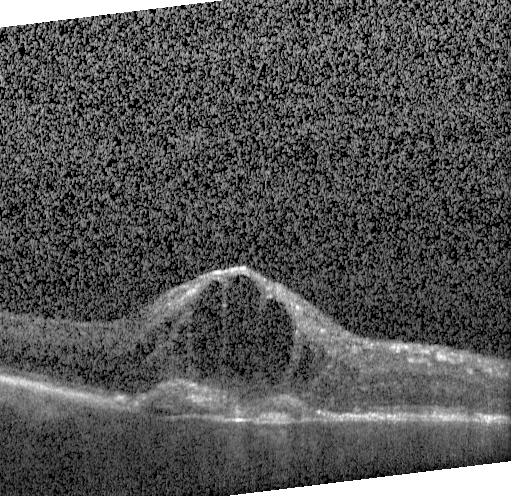 OCT finding: CNV.